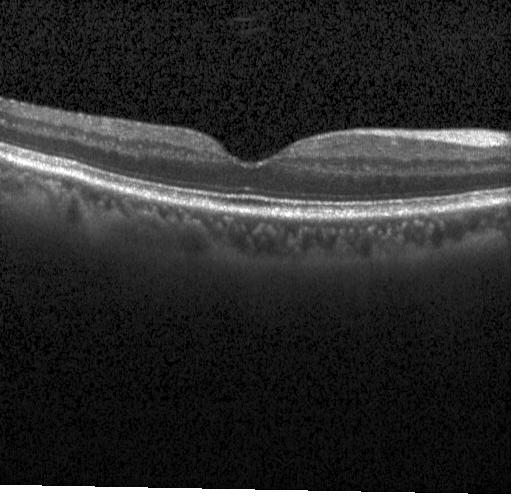 Through the macula, instrument: Heidelberg Spectralis, OCT line scan.
No choroidal neovascularization, diabetic macular edema, or drusen.